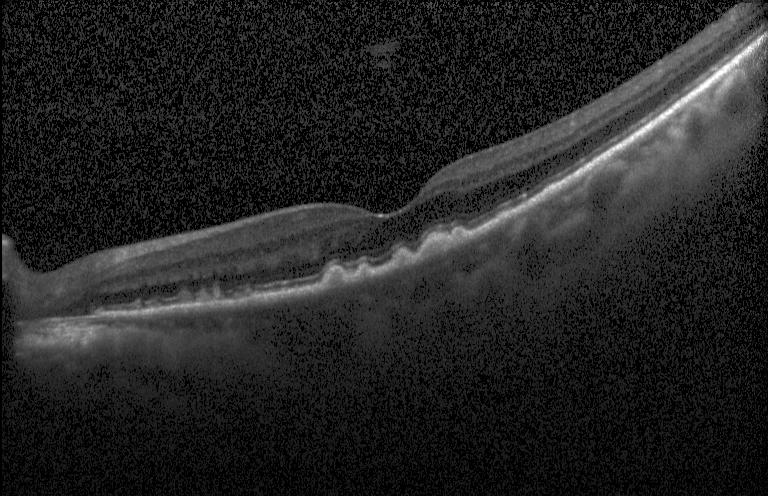

OCT scan showing sub-RPE drusenoid deposits.